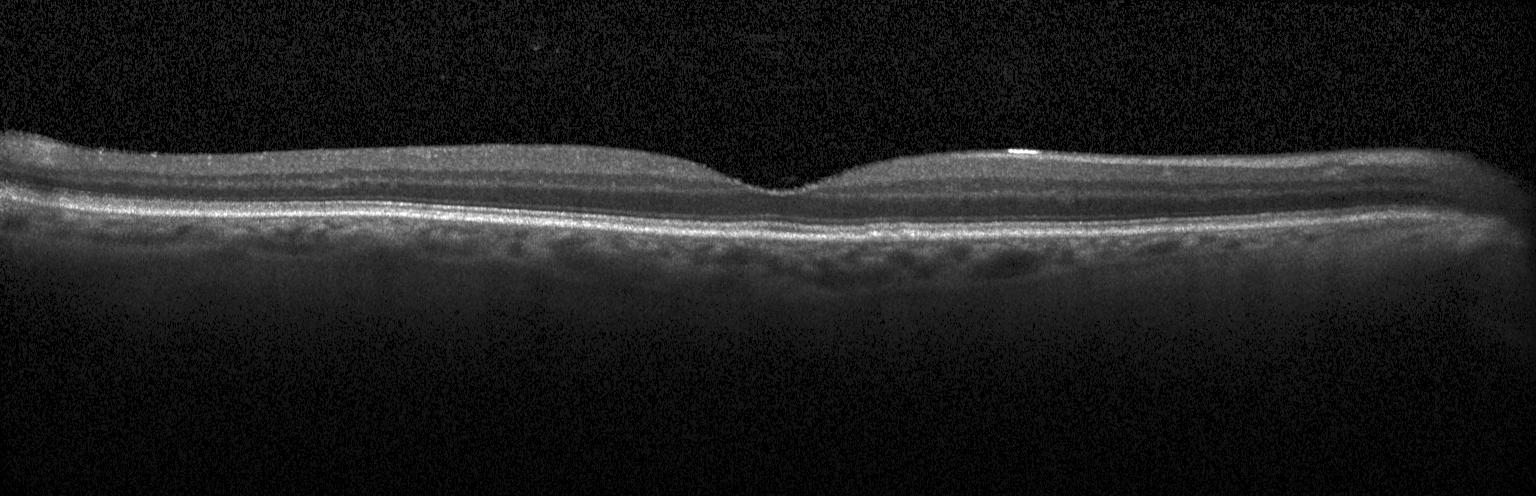
Retinal OCT cross-section, instrument: Heidelberg Spectralis — Diagnosis: no choroidal neovascularization, diabetic macular edema, or drusen.